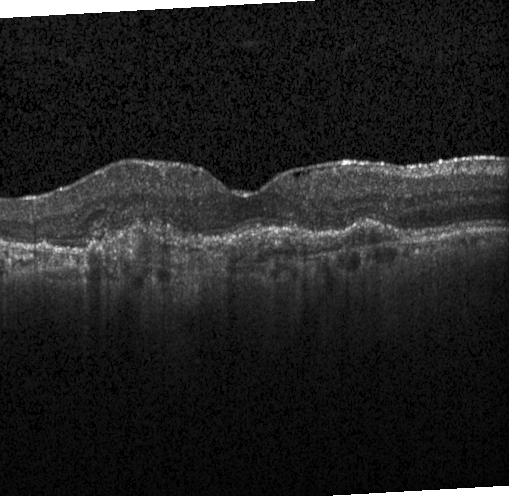

A choroidal neovascular membrane.